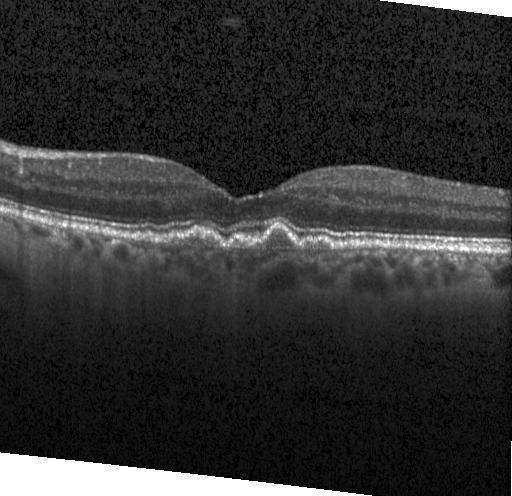 Macular scan. SD-OCT. Retinal OCT cross-section. Heidelberg Spectralis OCT system — Finding: drusen.